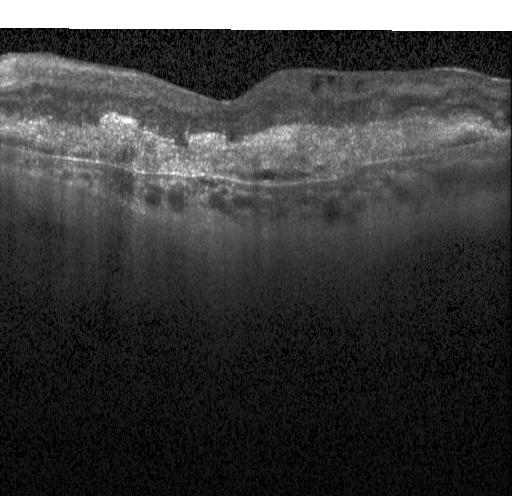

Macular OCT demonstrating a choroidal neovascular membrane.